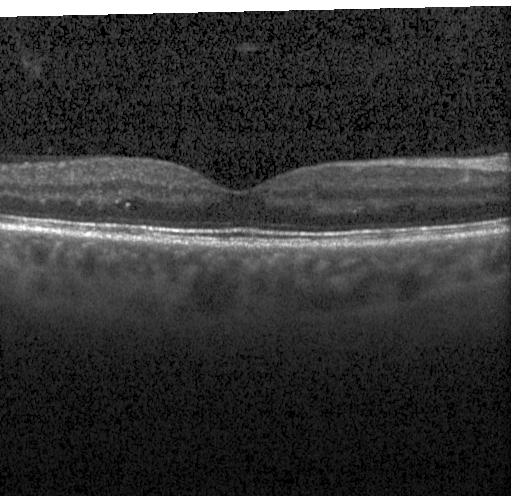 Acquired on a Heidelberg Spectralis · spectral-domain OCT · fovea-centered · retinal OCT cross-section.
Dx: no CNV, DME, or drusen.